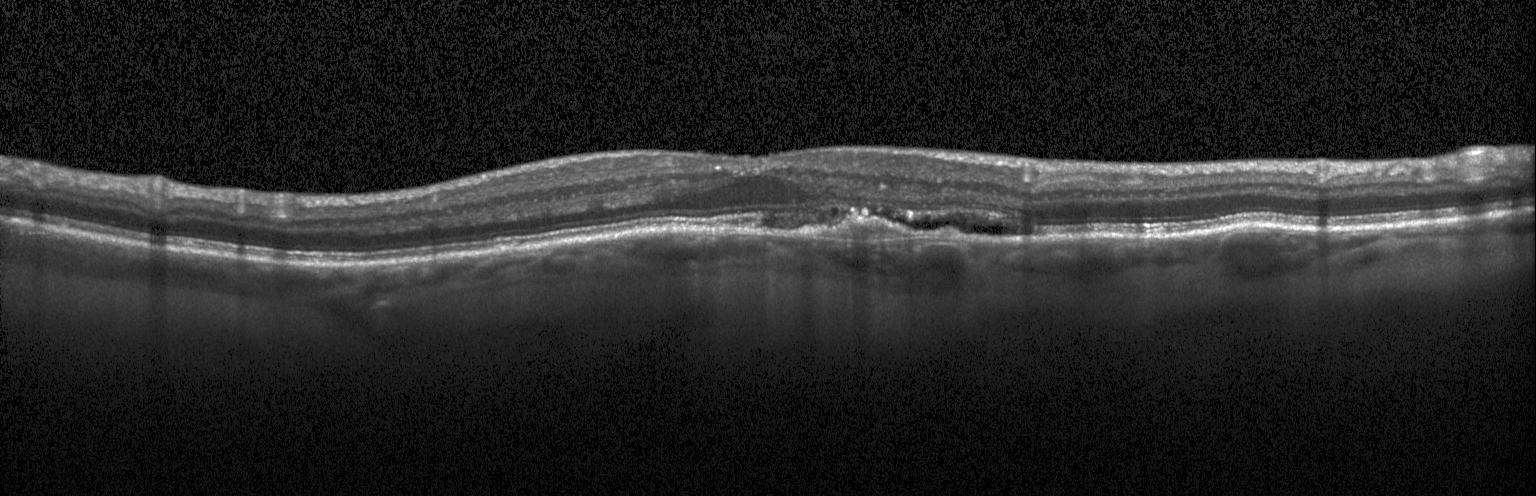

Diagnosis: choroidal neovascularization.